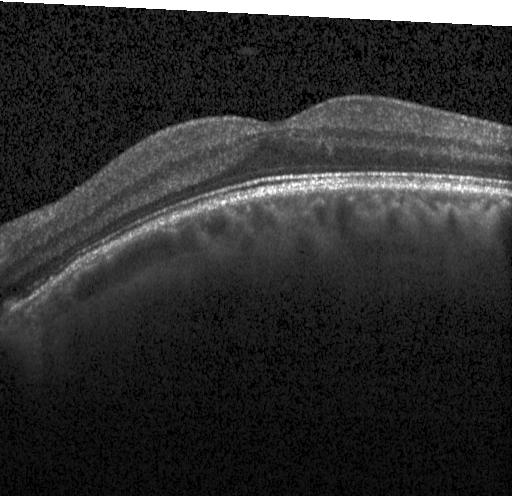 SD-OCT · Heidelberg Spectralis OCT system · OCT line scan
OCT finding: no evidence of choroidal neovascularization, diabetic macular edema, or drusen.